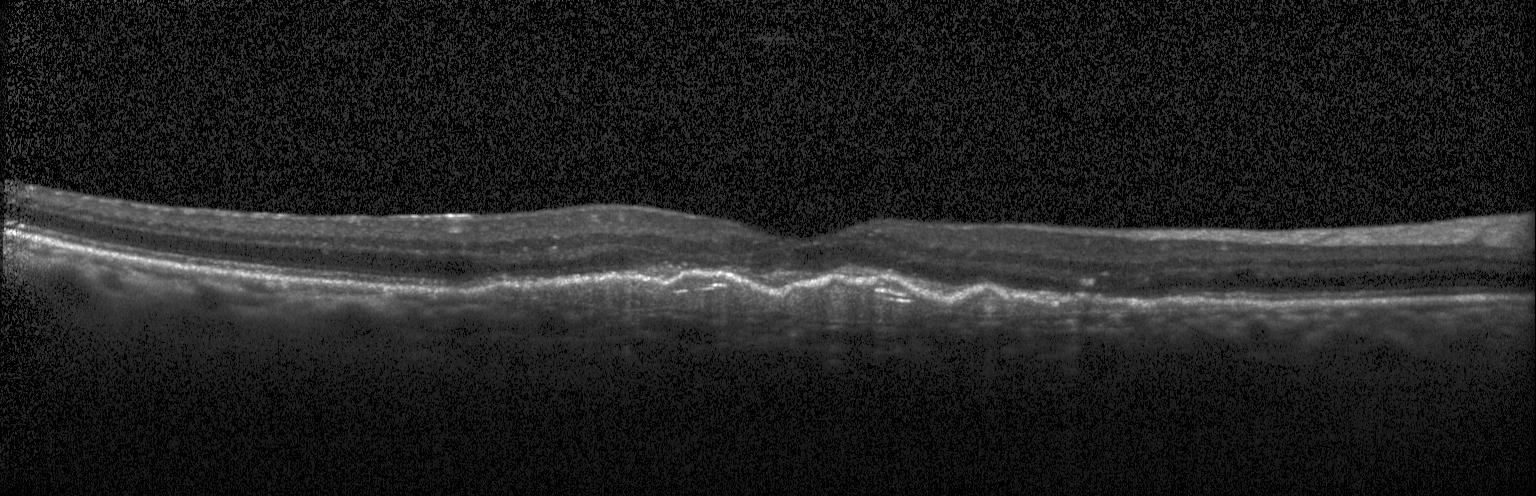
Spectral-domain OCT B-scan: a choroidal neovascular membrane.